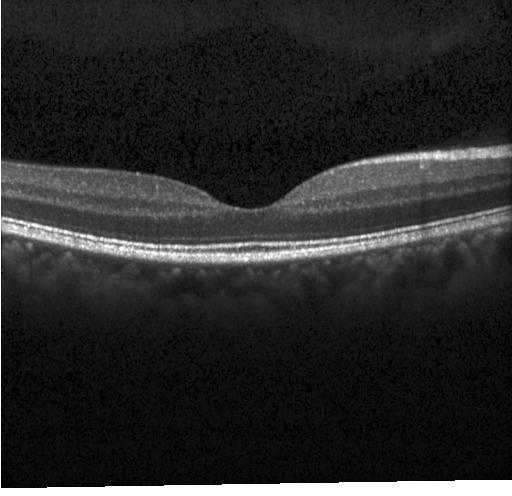 Retinal OCT cross-section — Finding: no CNV, no DME, and no drusen.